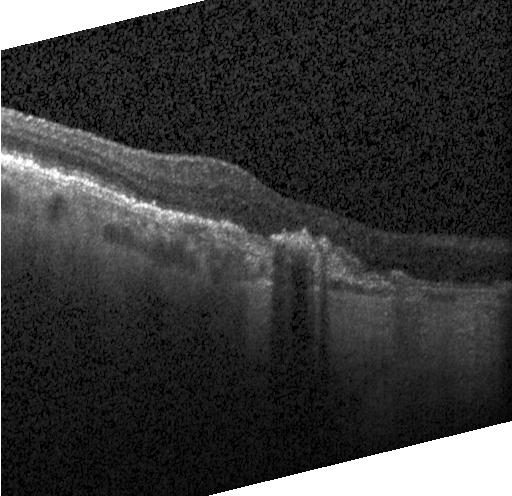 Finding: a choroidal neovascular membrane.